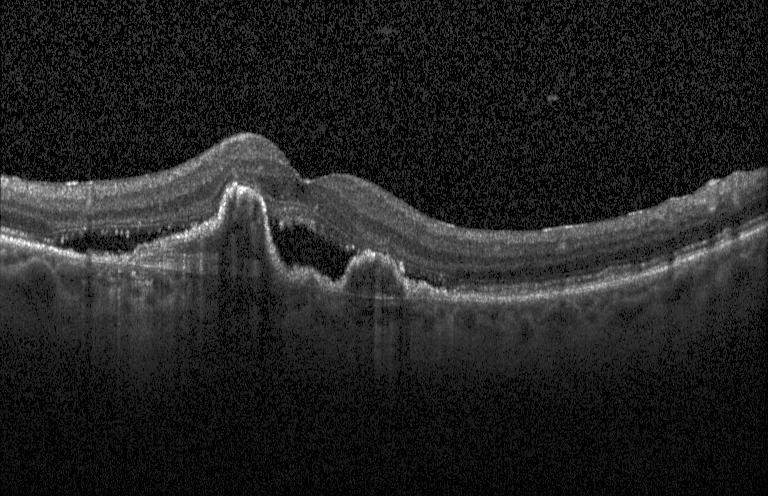
OCT finding: CNV.